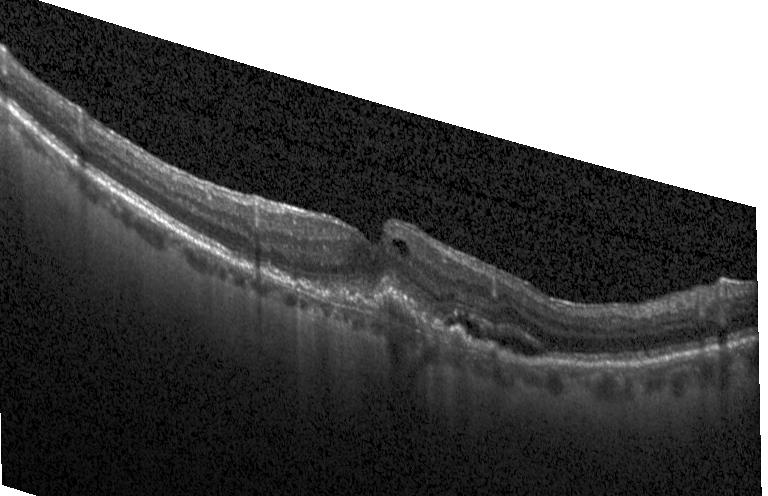

Centered on the fovea · optical coherence tomography B-scan · SD-OCT — Macular OCT: choroidal neovascularization (CNV).